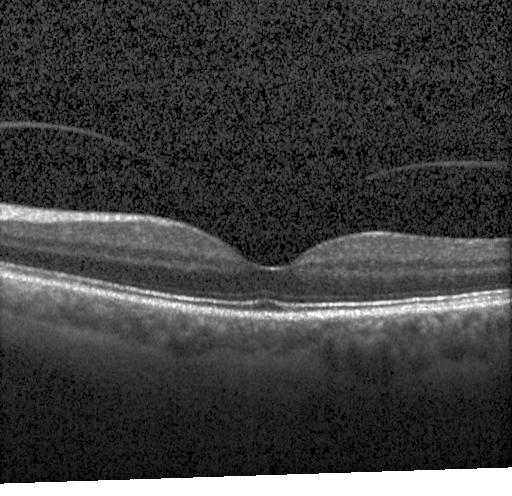
Optical coherence tomography scan. Spectral-domain optical coherence tomography.
The scan shows no evidence of CNV, DME, or drusen.